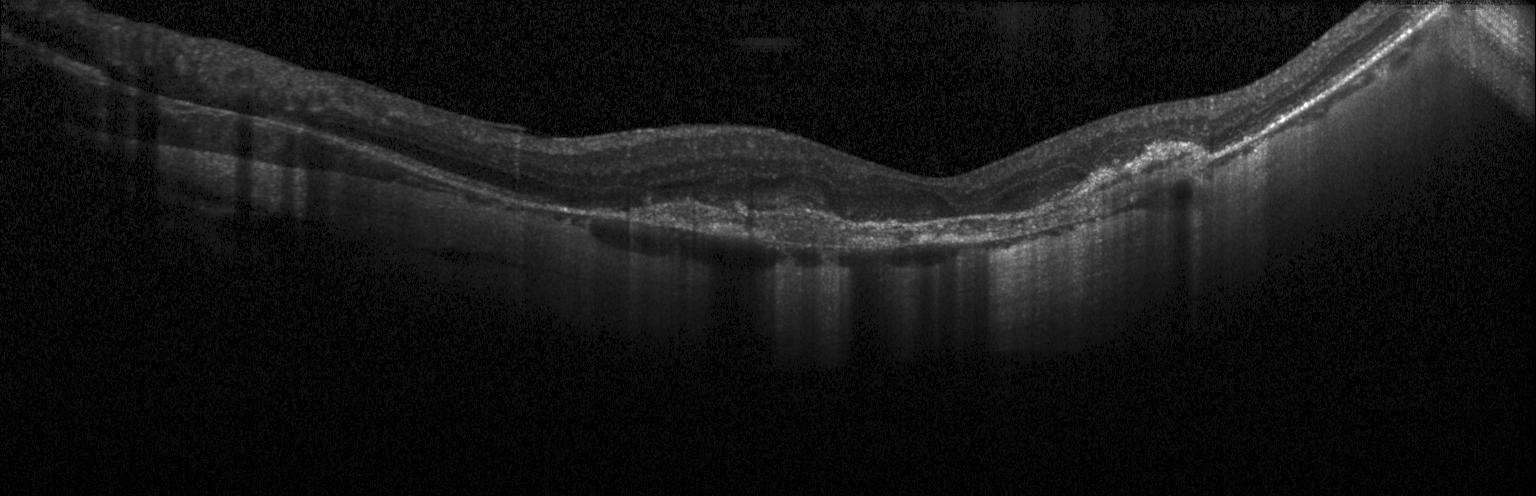

Acquired on a Heidelberg Spectralis, optical coherence tomography scan
Impression: CNV.